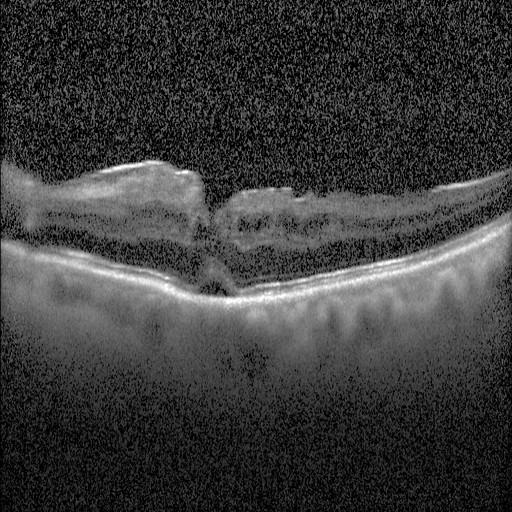

Impression: DME.